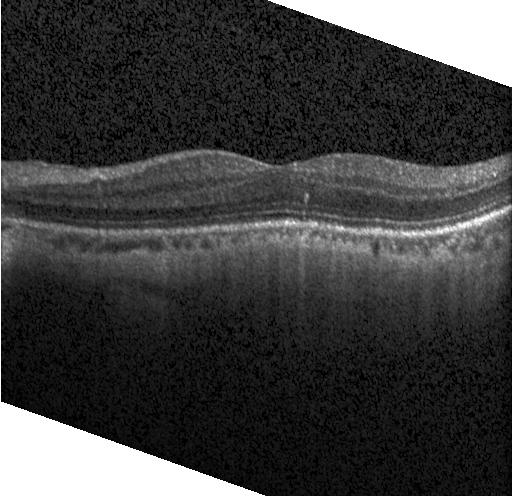
This B-scan demonstrates no evidence of choroidal neovascularization, diabetic macular edema, or drusen.